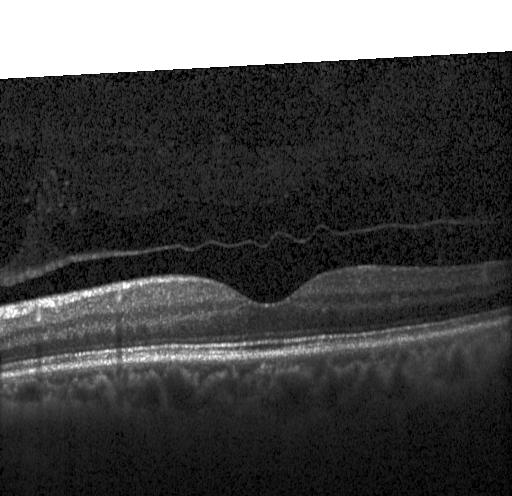 Retinal OCT cross-section showing neither choroidal neovascularization, diabetic macular edema, nor drusen.